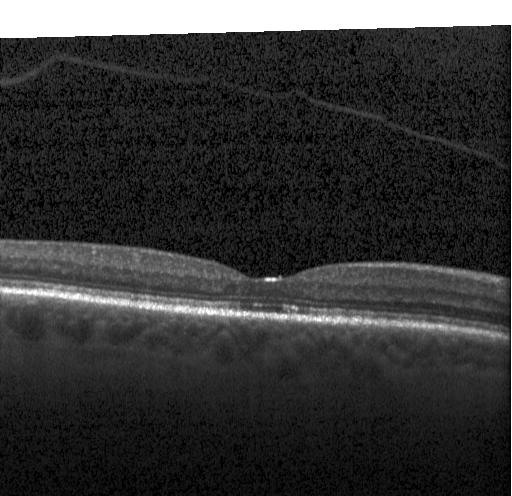

Optical coherence tomography B-scan.
Finding: no CNV, DME, or drusen.